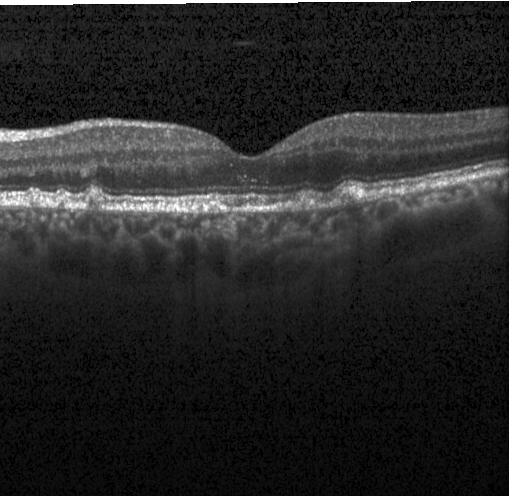 OCT finding: sub-RPE drusenoid deposits.